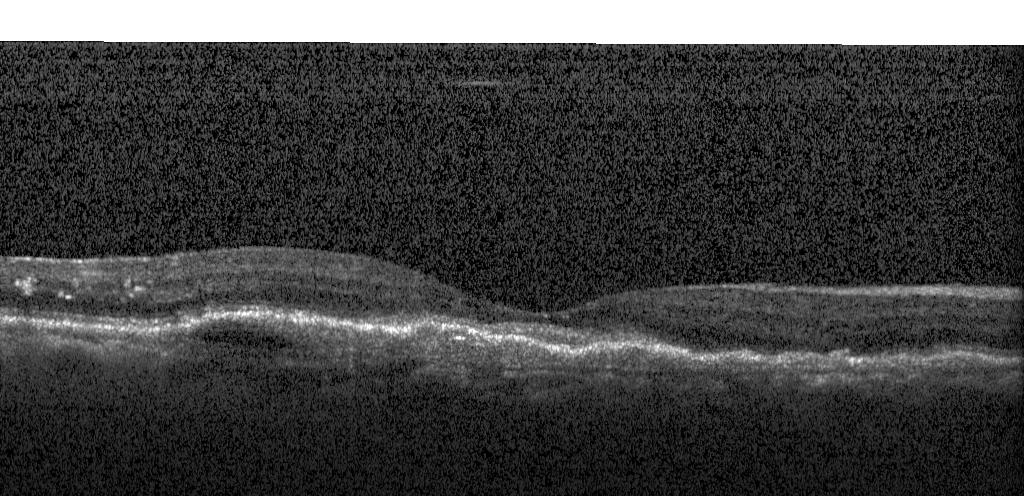
Optical coherence tomography B-scan
This B-scan demonstrates a choroidal neovascular membrane.